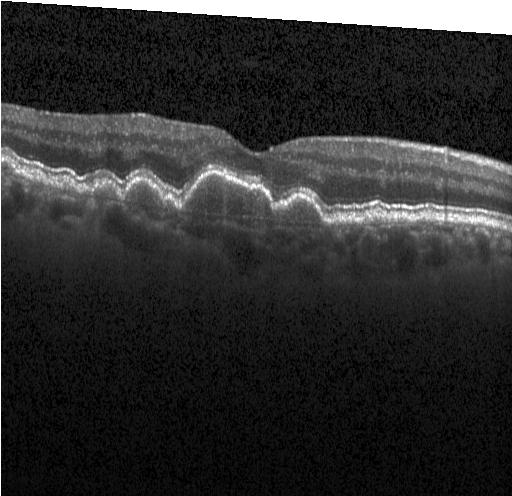

Instrument: Heidelberg Spectralis · horizontal scan through the fovea · spectral-domain OCT · OCT B-scan — Diagnosis: sub-RPE drusenoid deposits.